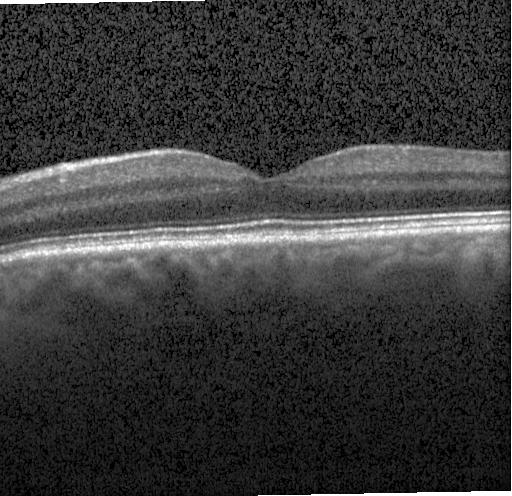
Fovea-centered; SD-OCT; optical coherence tomography B-scan; Heidelberg Spectralis. Dx: no choroidal neovascularization, no diabetic macular edema, and no drusen.